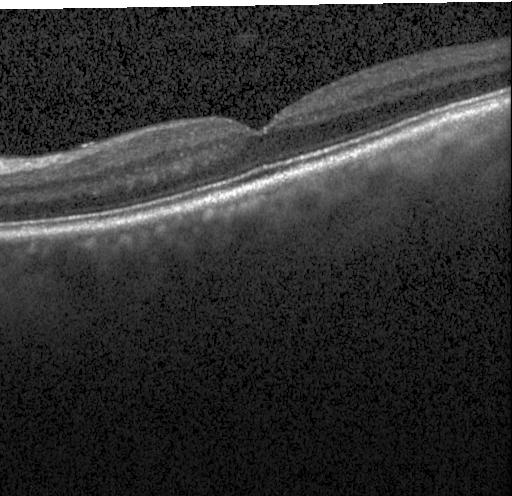

Fovea-centered, Heidelberg Spectralis, OCT B-scan — Impression: no evidence of CNV, DME, or drusen.